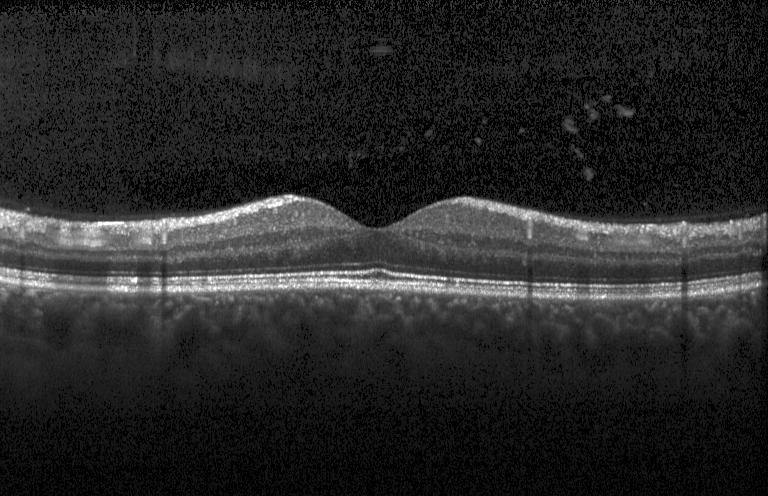

Macular OCT: no evidence of choroidal neovascularization, diabetic macular edema, or drusen.